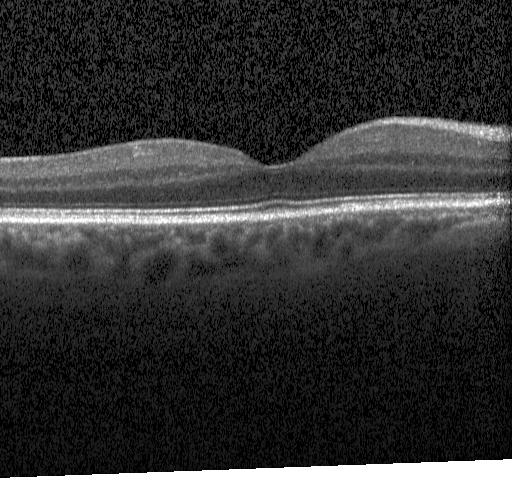
OCT scan showing neither CNV, DME, nor drusen.